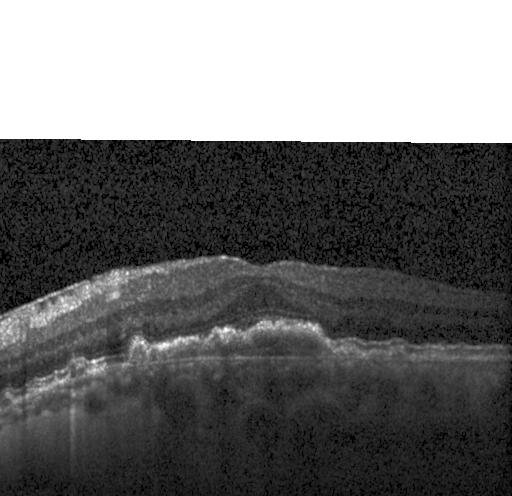 Retinal OCT B-scan — Diagnosis: a choroidal neovascular membrane.